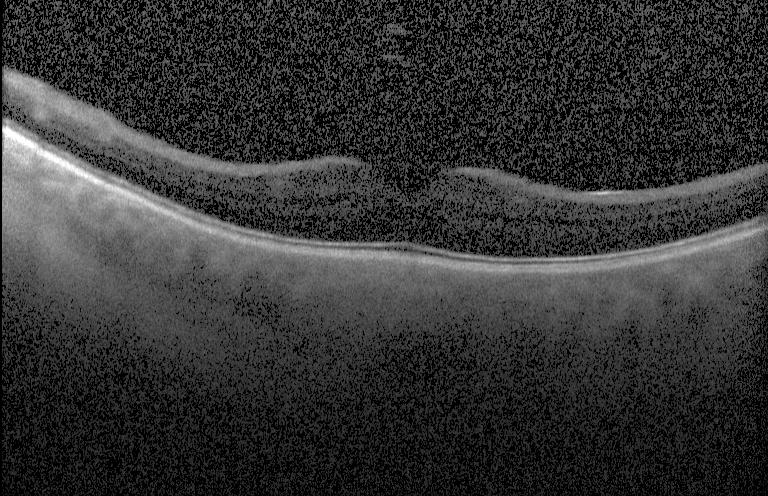 Impression: no CNV, no DME, and no drusen.